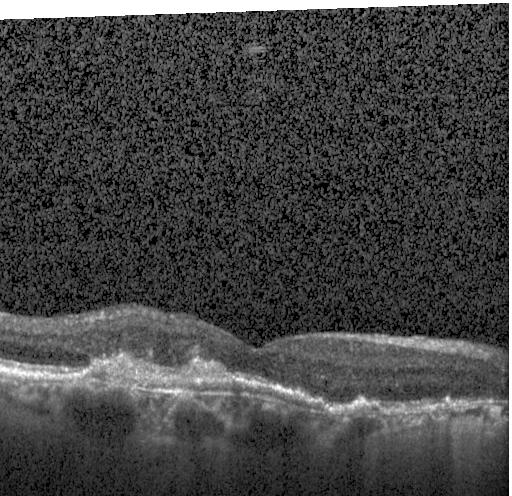 Horizontal scan through the fovea; instrument: Heidelberg Spectralis; retinal OCT B-scan
Assessment: a choroidal neovascular membrane.